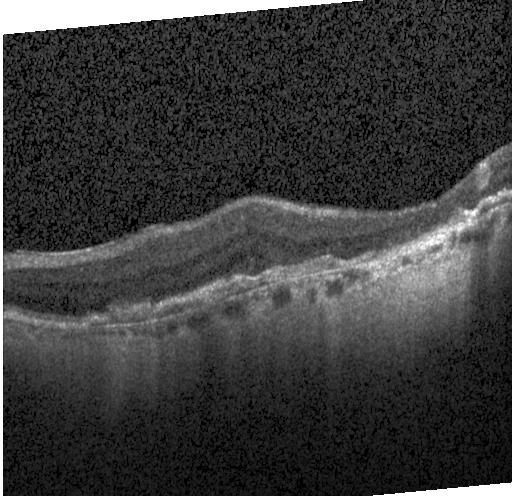

Heidelberg Spectralis OCT system, retinal OCT cross-section.
Assessment: a choroidal neovascular membrane.